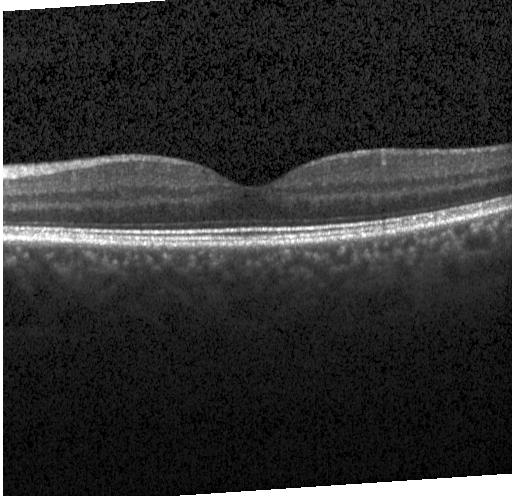

Retinal OCT cross-section — Impression: no evidence of CNV, DME, or drusen.